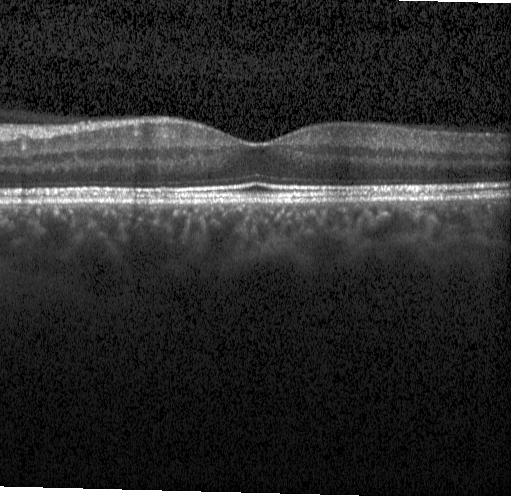
Horizontal scan through the fovea. OCT line scan
Finding: no choroidal neovascularization, diabetic macular edema, or drusen.